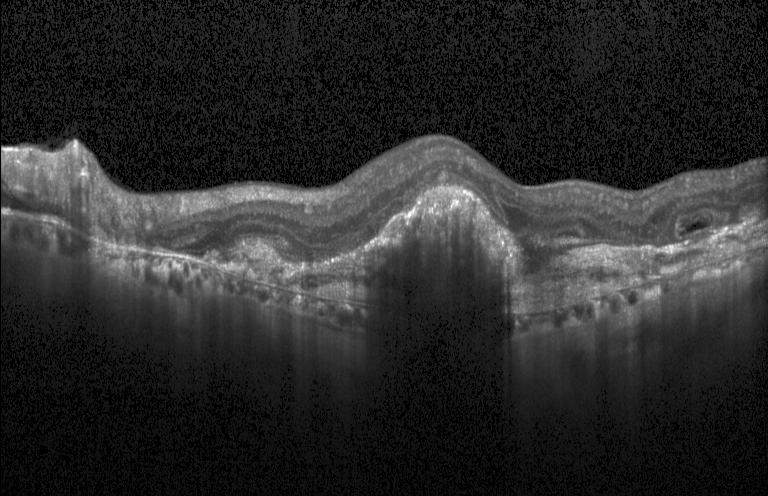

OCT scan showing a choroidal neovascular membrane.